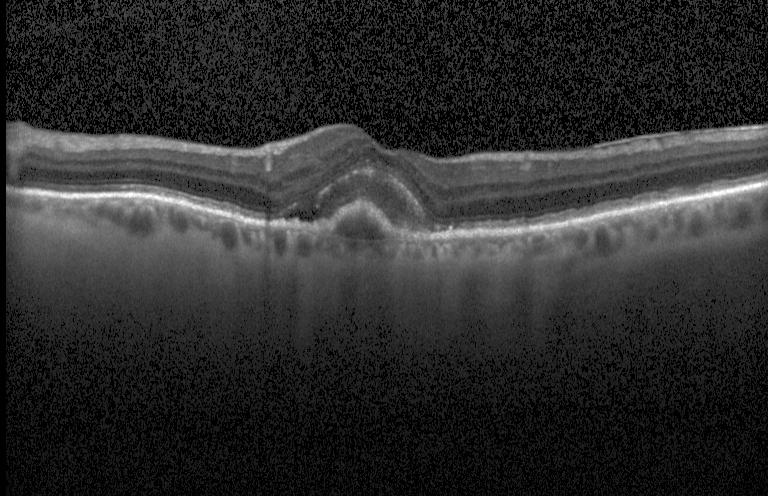
Finding: a choroidal neovascular membrane.